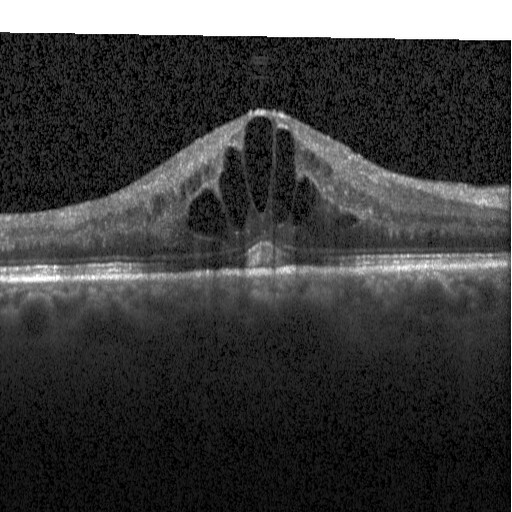
Impression: diabetic macular edema.